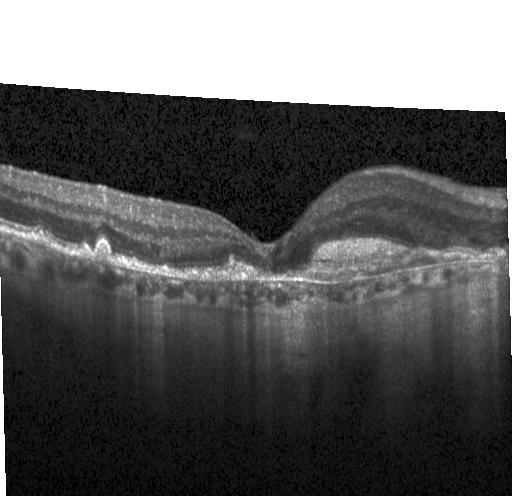 Impression: a choroidal neovascular membrane.